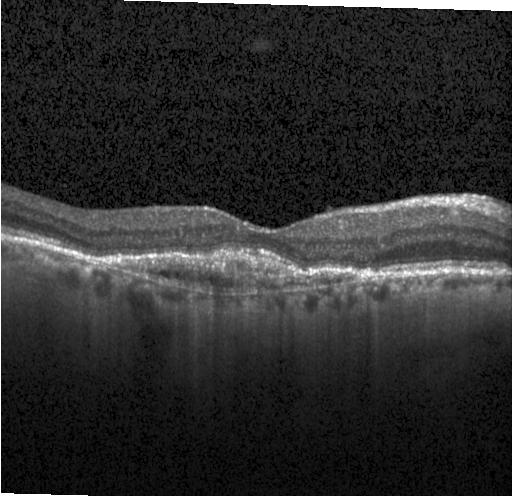
Diagnosis: a choroidal neovascular membrane.